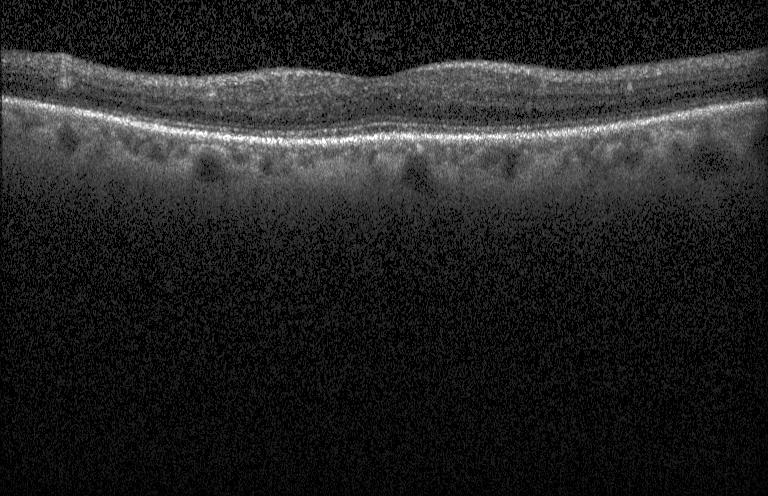 Assessment: no CNV, no DME, and no drusen.